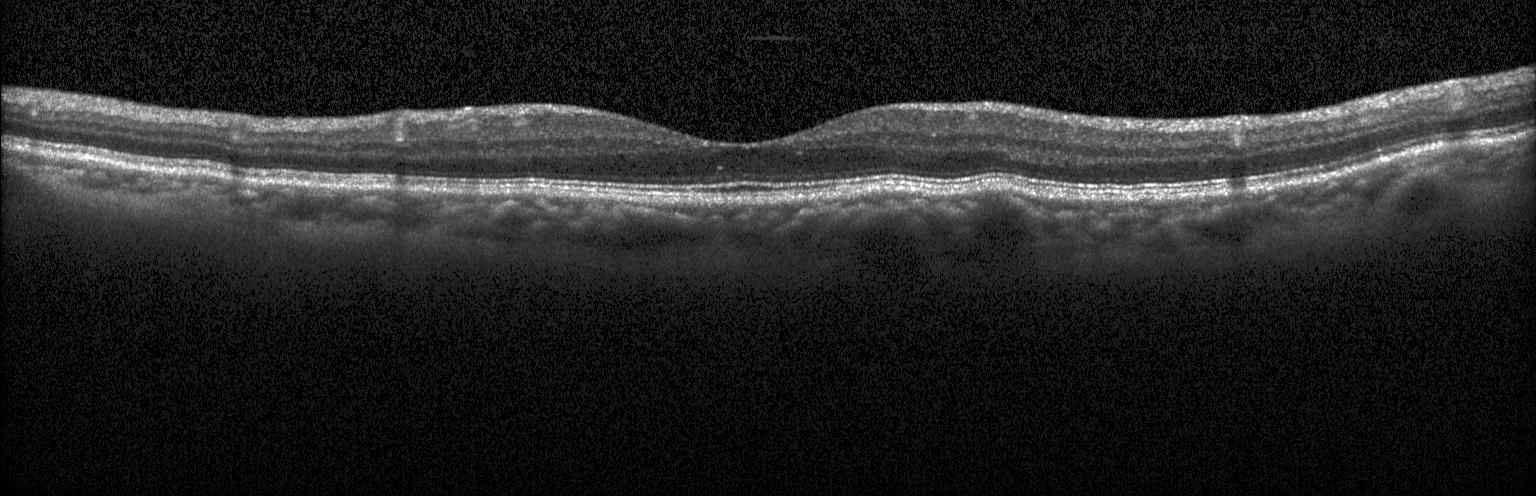

Spectral-domain optical coherence tomography, OCT line scan
Impression: multiple drusen.